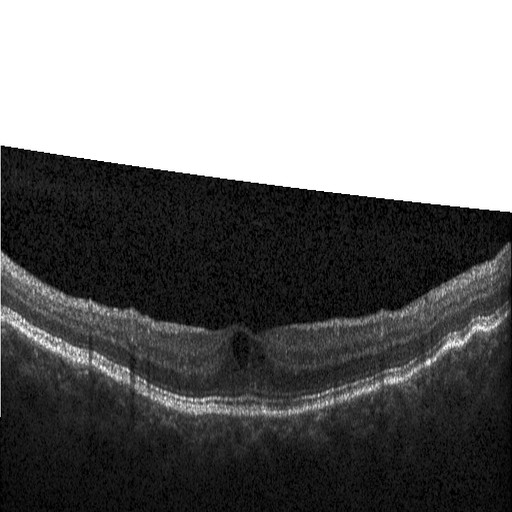

This B-scan demonstrates DME.